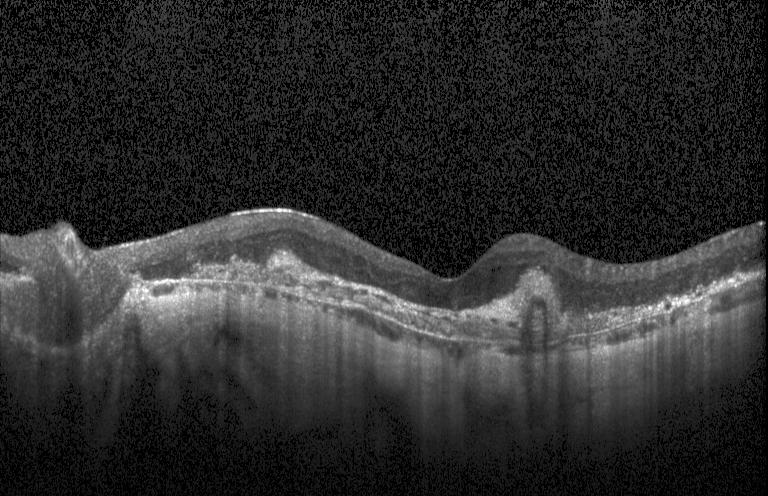

OCT B-scan · acquired on a Heidelberg Spectralis — OCT finding: a choroidal neovascular membrane.